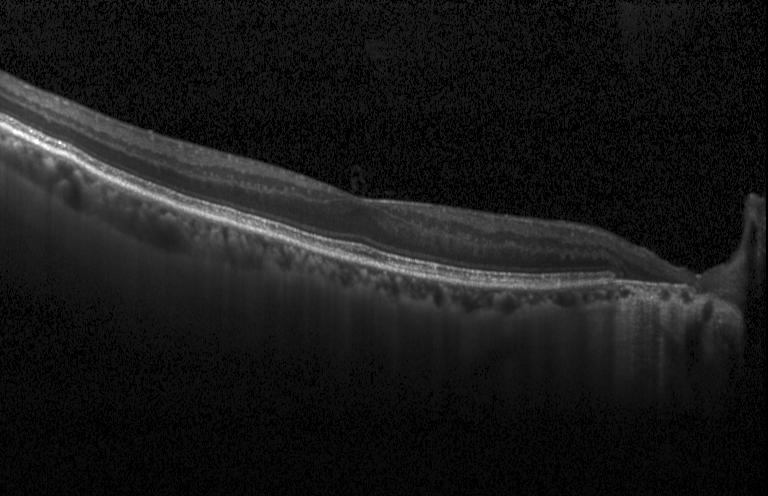 Optical coherence tomography B-scan, spectral-domain optical coherence tomography, Heidelberg Spectralis, horizontal scan through the fovea
The scan shows no choroidal neovascularization, no diabetic macular edema, and no drusen.